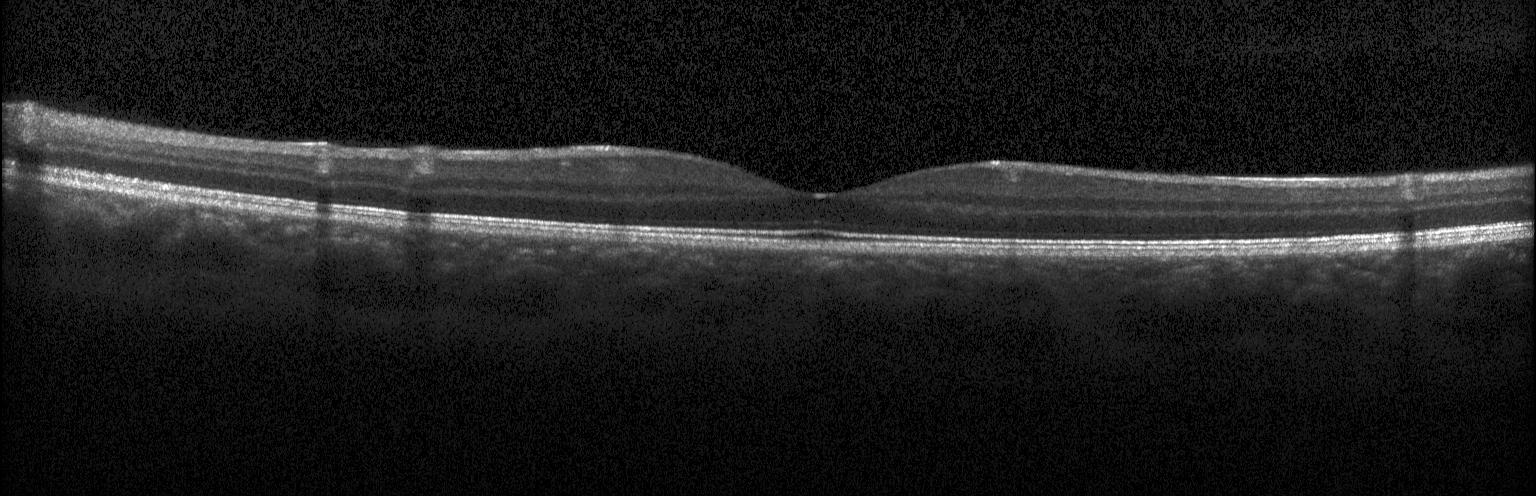

Acquired on a Heidelberg Spectralis · through the macula · spectral-domain optical coherence tomography · optical coherence tomography scan
Macular OCT: no choroidal neovascularization, no diabetic macular edema, and no drusen.